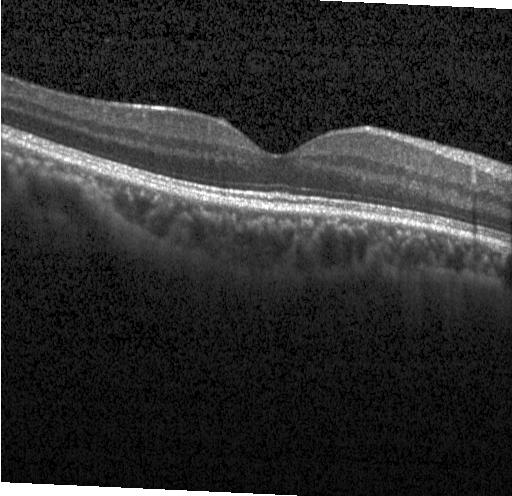
Optical coherence tomography B-scan; fovea-centered; spectral-domain optical coherence tomography
Finding: no choroidal neovascularization, no diabetic macular edema, and no drusen.